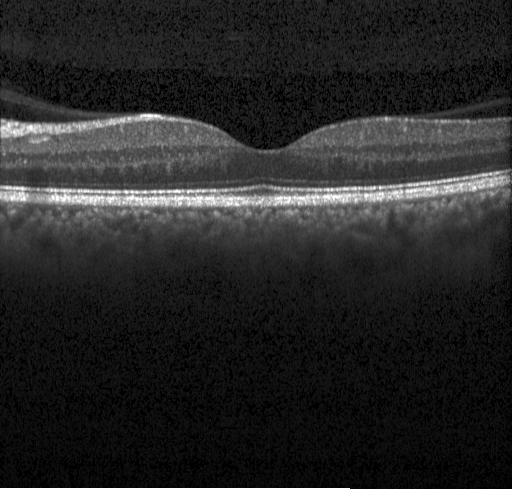
Optical coherence tomography B-scan. Spectral-domain OCT. Macular scan. Heidelberg Spectralis
Dx: no evidence of choroidal neovascularization, diabetic macular edema, or drusen.